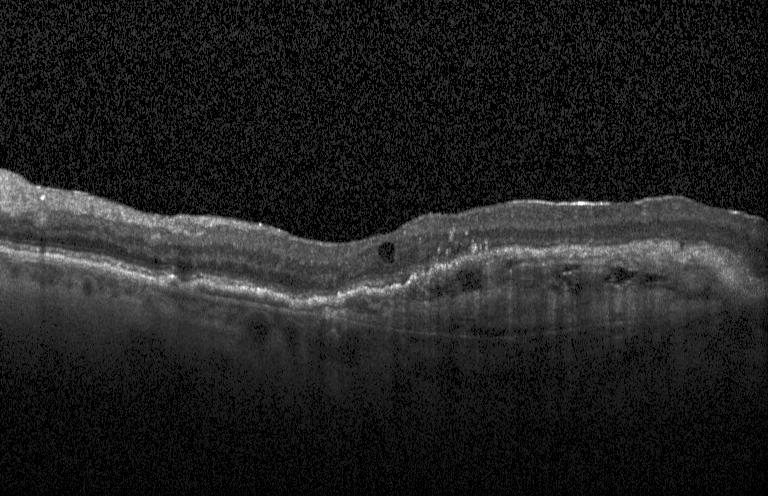
OCT B-scan showing choroidal neovascularization (CNV).